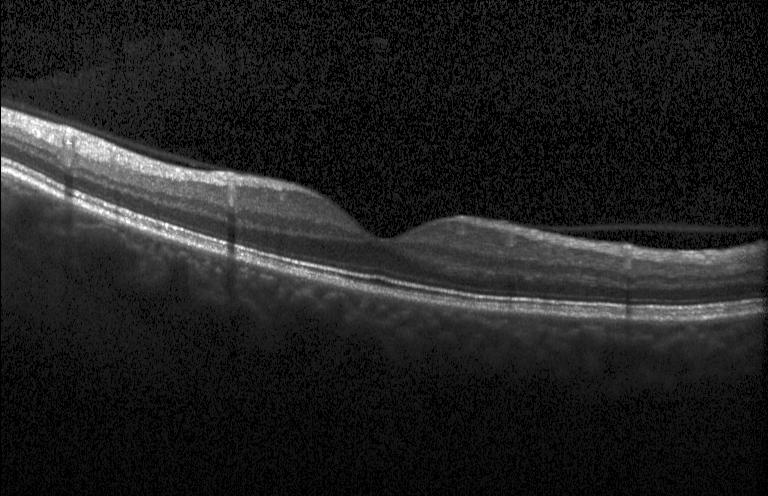

OCT scan showing no choroidal neovascularization, no diabetic macular edema, and no drusen.